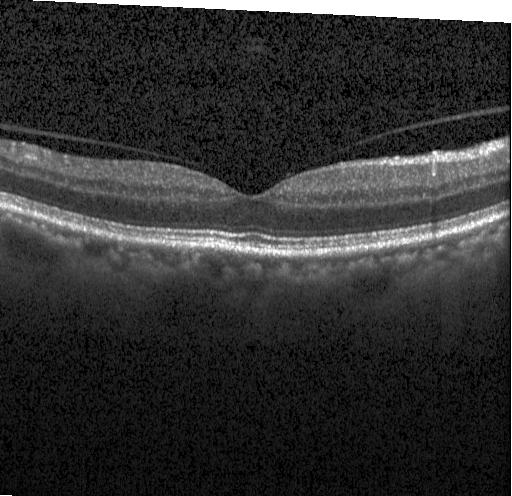
OCT line scan. Assessment: neither choroidal neovascularization, diabetic macular edema, nor drusen.